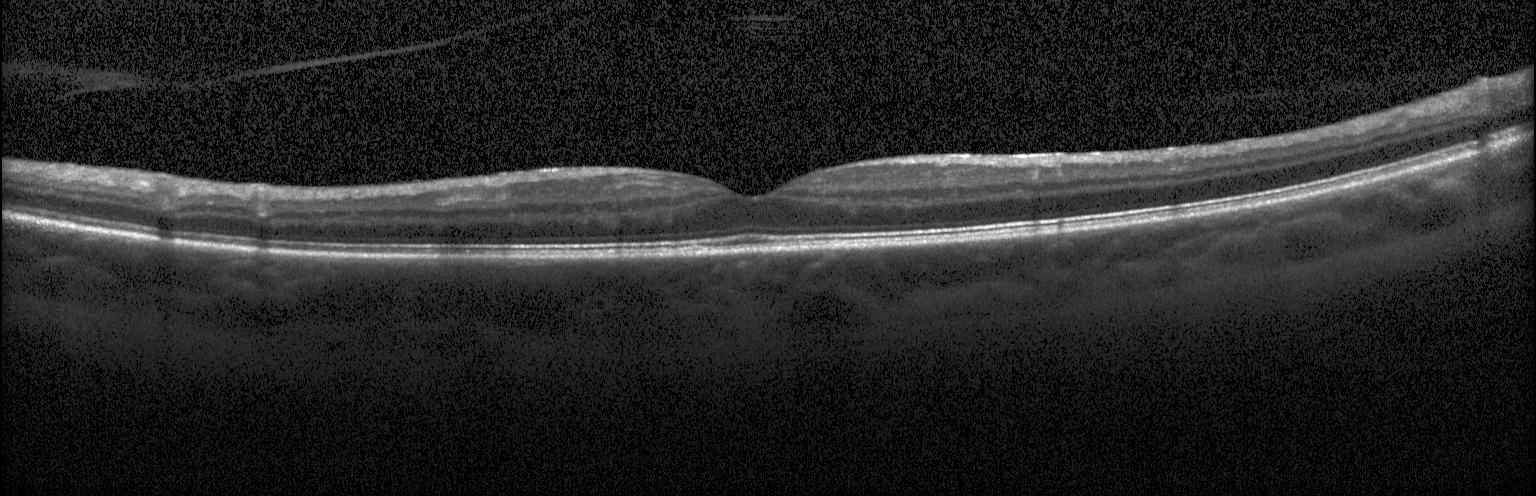

Spectral-domain OCT B-scan: no choroidal neovascularization, no diabetic macular edema, and no drusen.